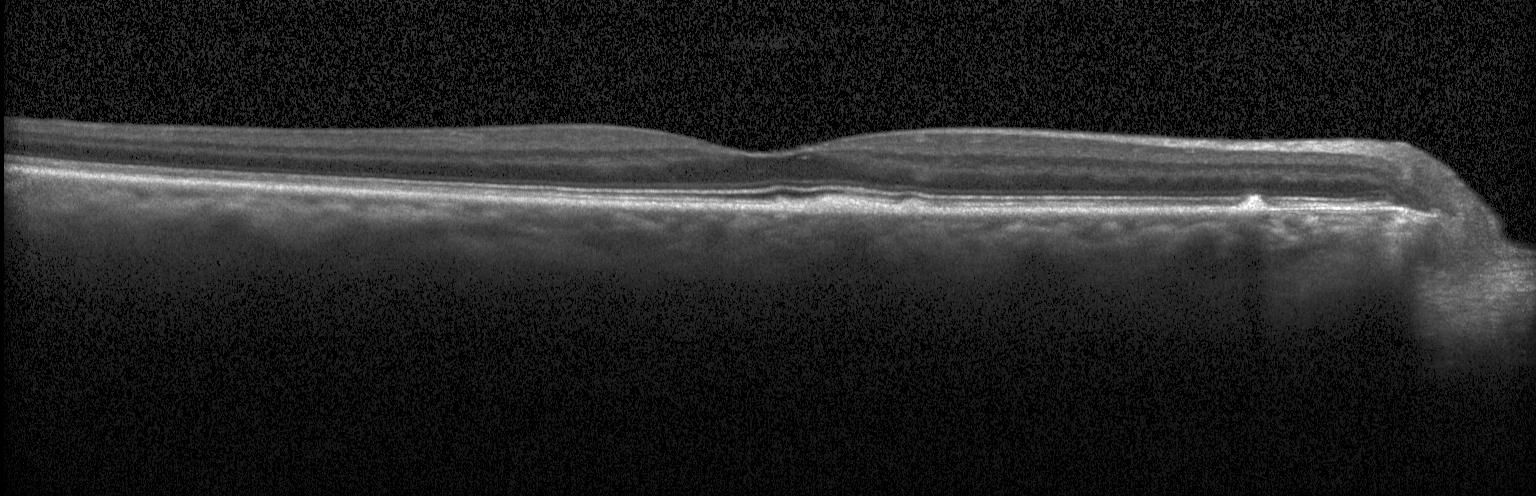

Finding: drusen.